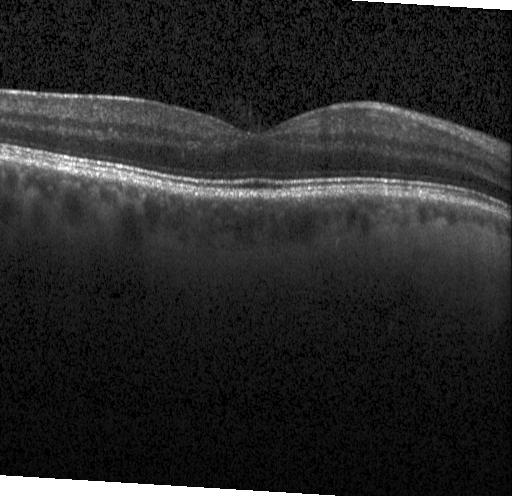
Retinal OCT B-scan · Heidelberg Spectralis. The scan shows no evidence of CNV, DME, or drusen.